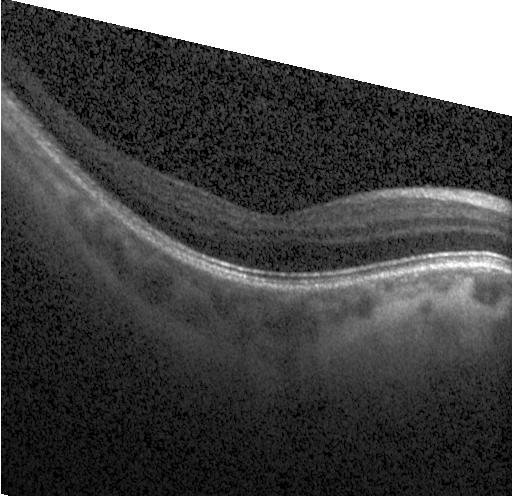 Heidelberg Spectralis OCT system · spectral-domain optical coherence tomography · fovea-centered · optical coherence tomography B-scan
Finding: no choroidal neovascularization, no diabetic macular edema, and no drusen.